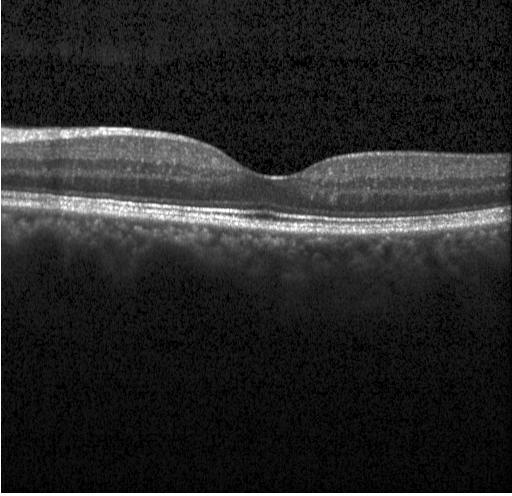
Spectral-domain optical coherence tomography · retinal OCT cross-section · acquired on a Heidelberg Spectralis
Diagnosis: neither CNV, DME, nor drusen.